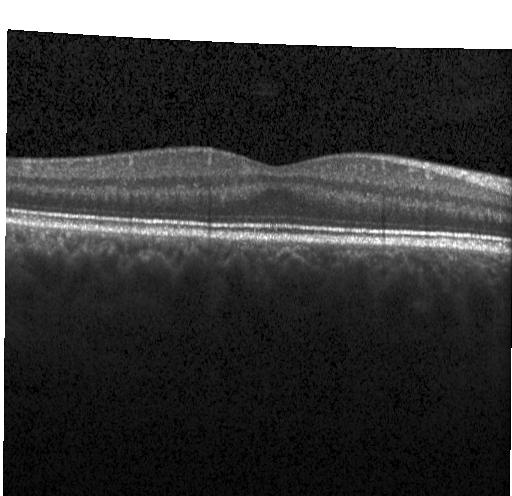 Macular scan; optical coherence tomography scan — Assessment: no choroidal neovascularization, diabetic macular edema, or drusen.